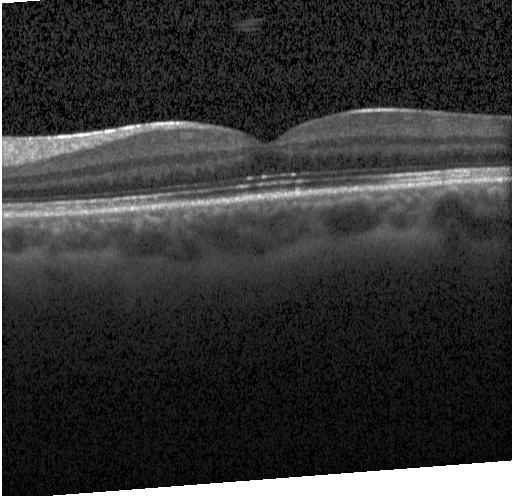 OCT finding: neither choroidal neovascularization, diabetic macular edema, nor drusen.